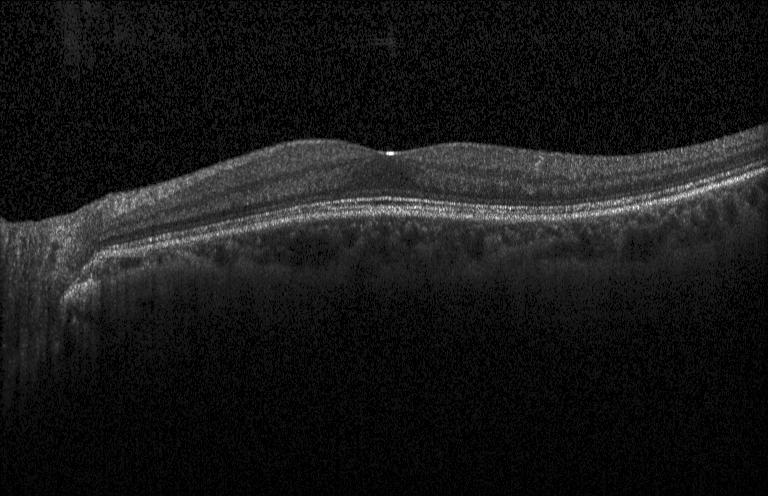 OCT B-scan.
Diagnosis: no CNV, DME, or drusen.